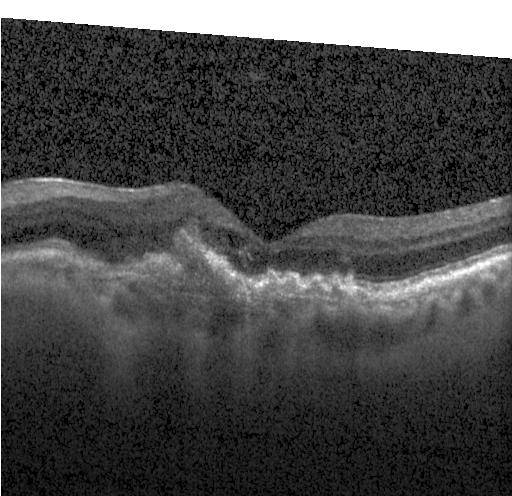 Instrument: Heidelberg Spectralis, retinal OCT B-scan, fovea-centered — Finding: CNV.